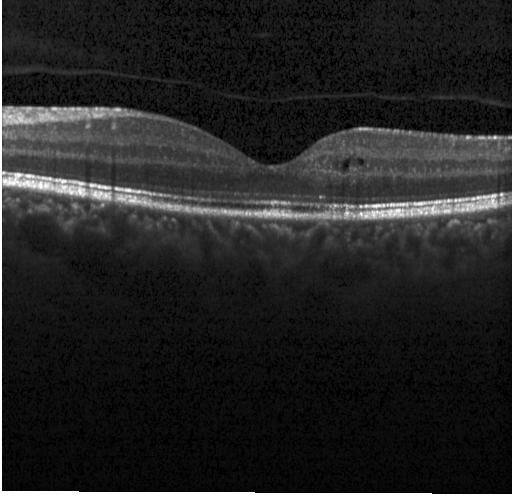
OCT B-scan, Heidelberg Spectralis, macular scan
Assessment: diabetic macular edema (DME).